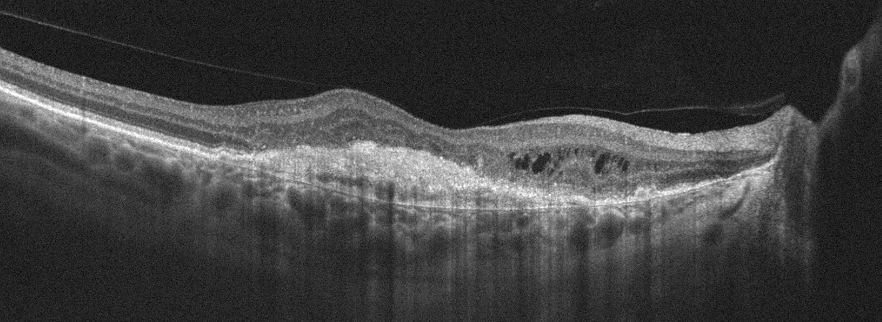

OCT B-scan. OD.
Age-related macular degeneration.